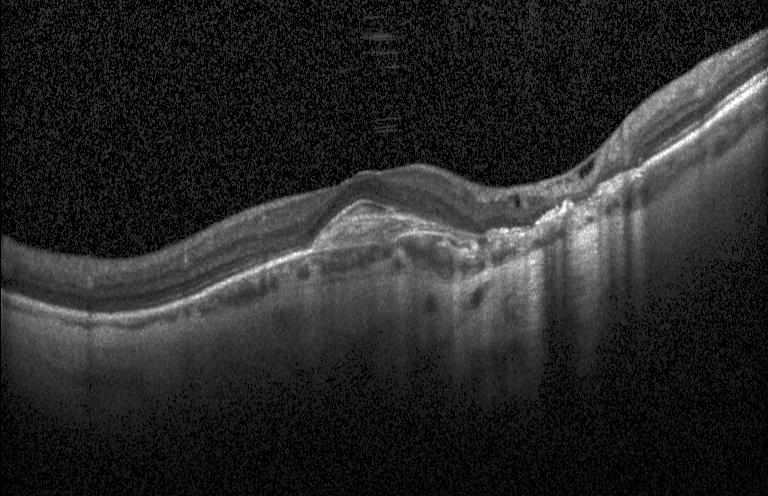 OCT B-scan, centered on the fovea, spectral-domain optical coherence tomography
A choroidal neovascular membrane.